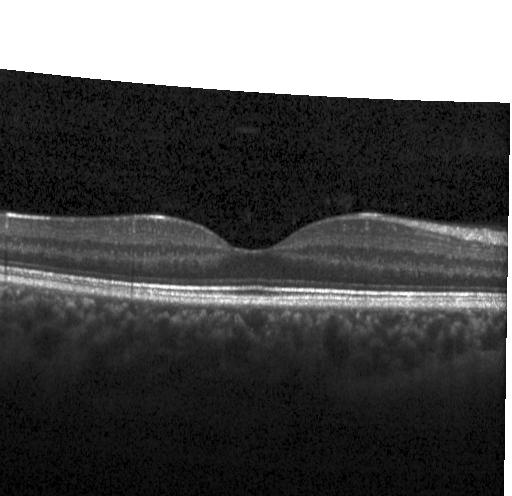
Retinal OCT cross-section, macular scan, Heidelberg Spectralis OCT system. Assessment: neither choroidal neovascularization, diabetic macular edema, nor drusen.